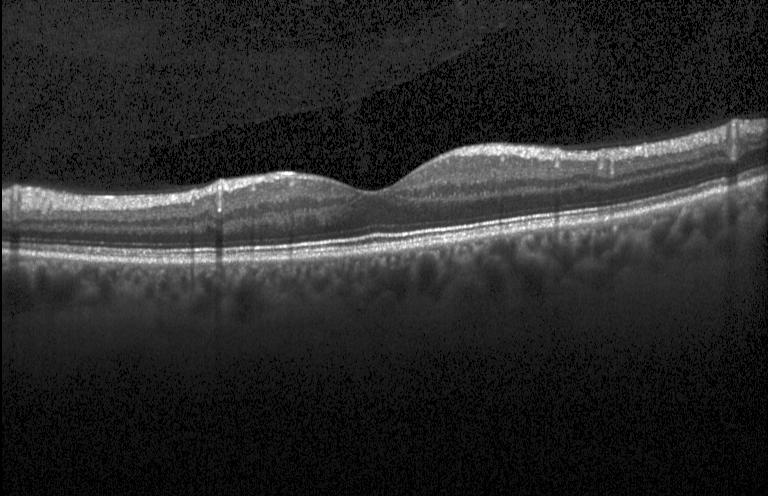 Horizontal scan through the fovea; spectral-domain optical coherence tomography; retinal OCT cross-section; instrument: Heidelberg Spectralis — Finding: no CNV, no DME, and no drusen.